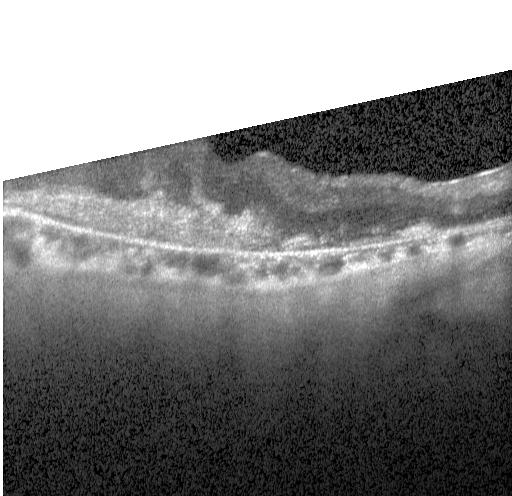
Optical coherence tomography B-scan.
This B-scan demonstrates choroidal neovascularization.